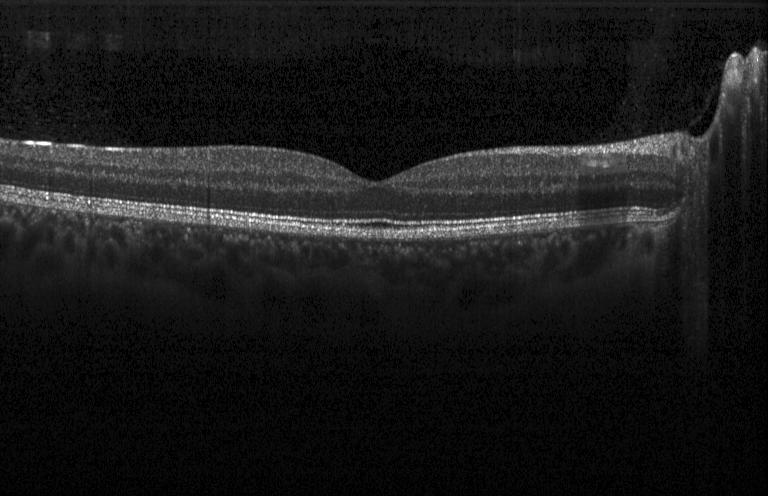
Finding: no CNV, no DME, and no drusen.